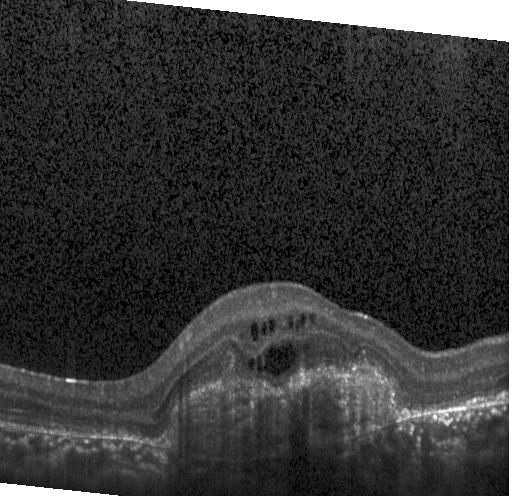 Optical coherence tomography scan · spectral-domain optical coherence tomography · Heidelberg Spectralis OCT system · macular scan — Macular OCT: choroidal neovascularization.